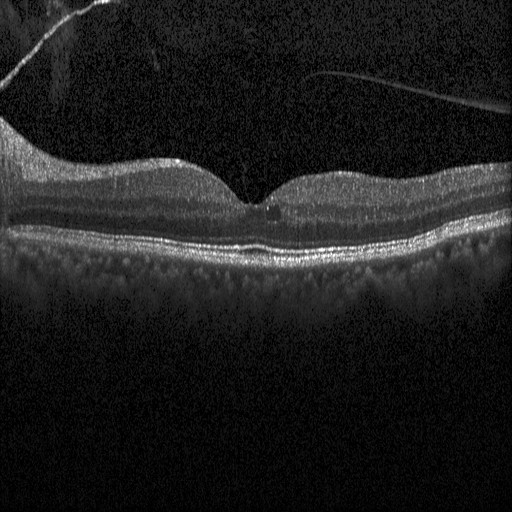
Instrument: Heidelberg Spectralis, retinal OCT B-scan, spectral-domain optical coherence tomography, through the macula
The scan shows diabetic macular edema (DME).